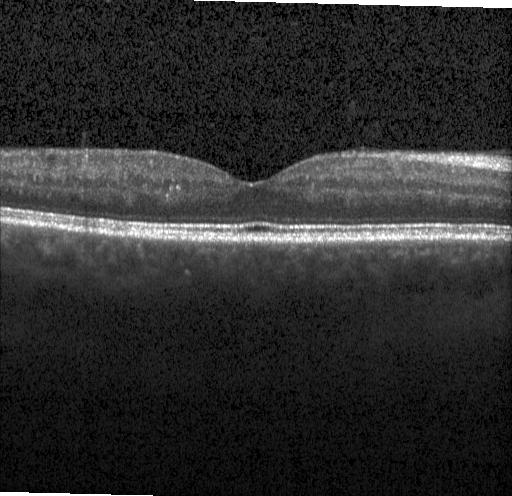
Spectral-domain OCT B-scan: no evidence of choroidal neovascularization, diabetic macular edema, or drusen.